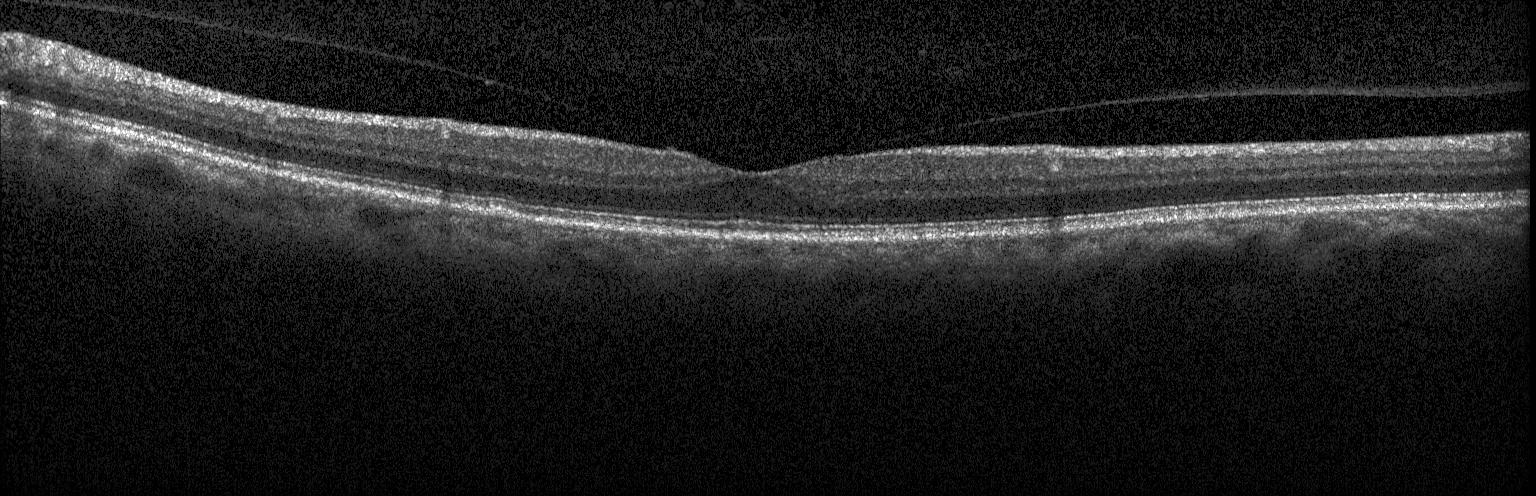
Optical coherence tomography scan
The scan shows no choroidal neovascularization, diabetic macular edema, or drusen.